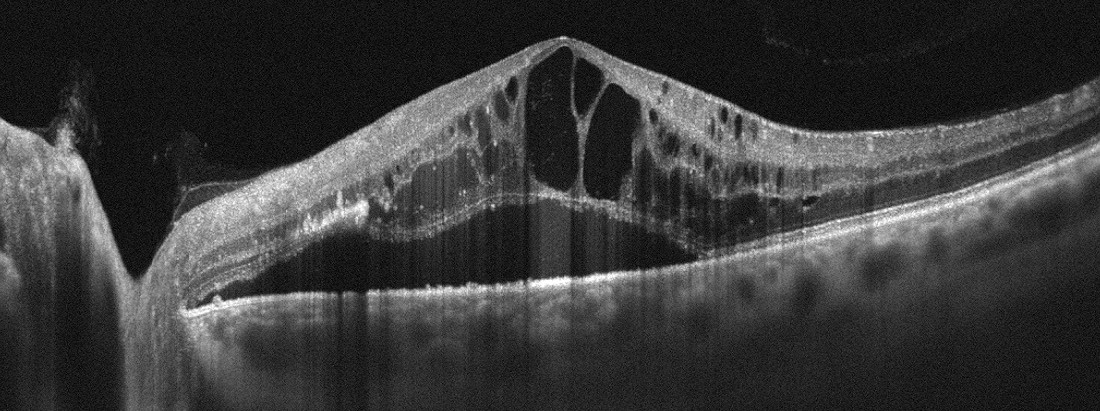

Impression: retinal vein occlusion.